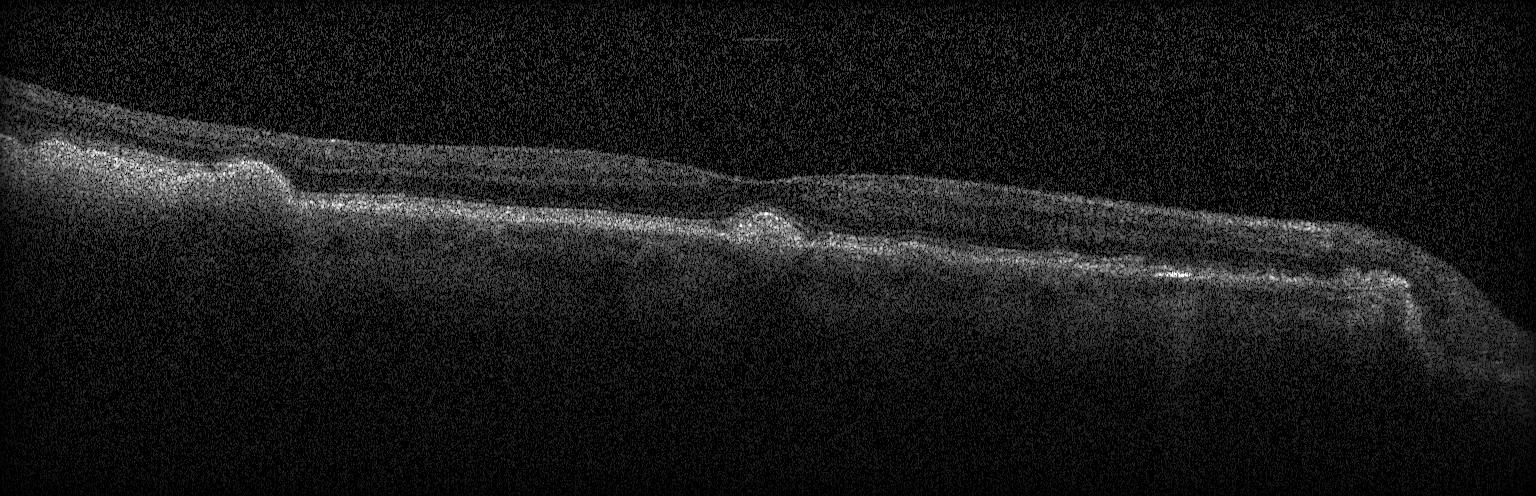

OCT line scan. The scan shows drusen.